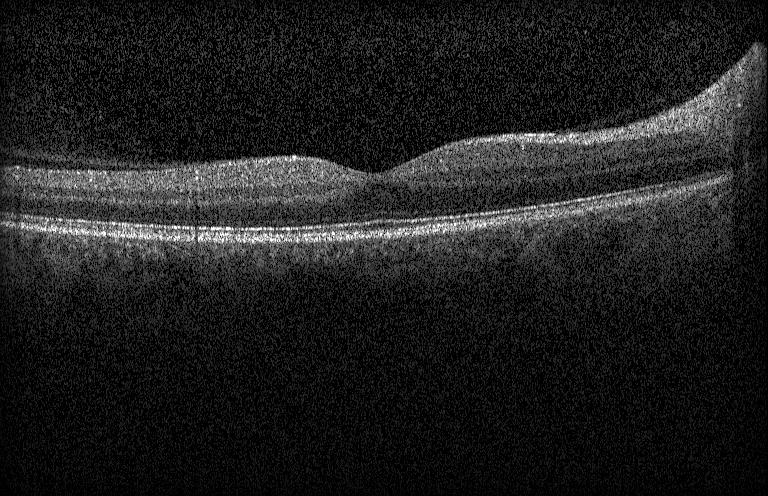 Retinal OCT cross-section — The scan shows neither CNV, DME, nor drusen.